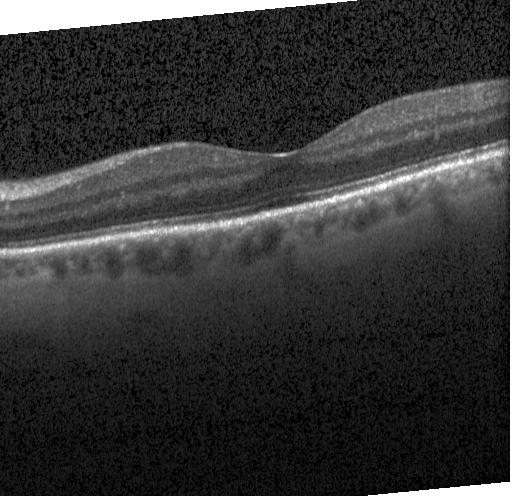

Impression: no choroidal neovascularization, no diabetic macular edema, and no drusen.